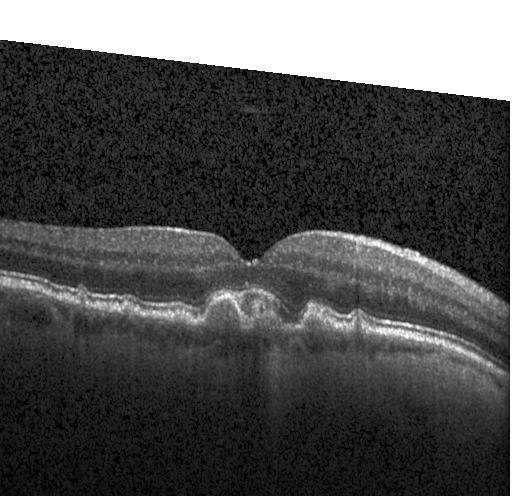
Spectral-domain OCT · Heidelberg Spectralis · fovea-centered · retinal OCT cross-section — Finding: sub-RPE drusenoid deposits.